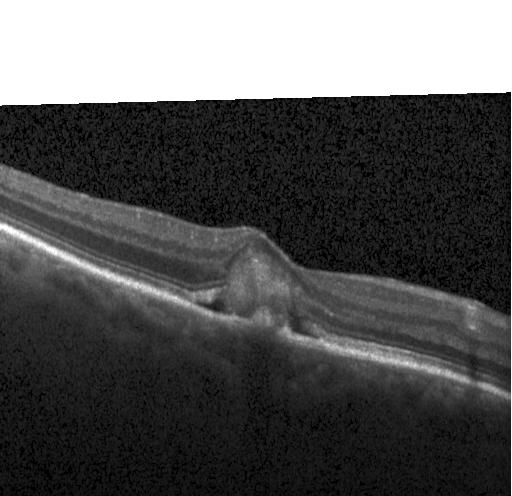
Optical coherence tomography B-scan. Acquired on a Heidelberg Spectralis. Macular scan — Diagnosis: a choroidal neovascular membrane.